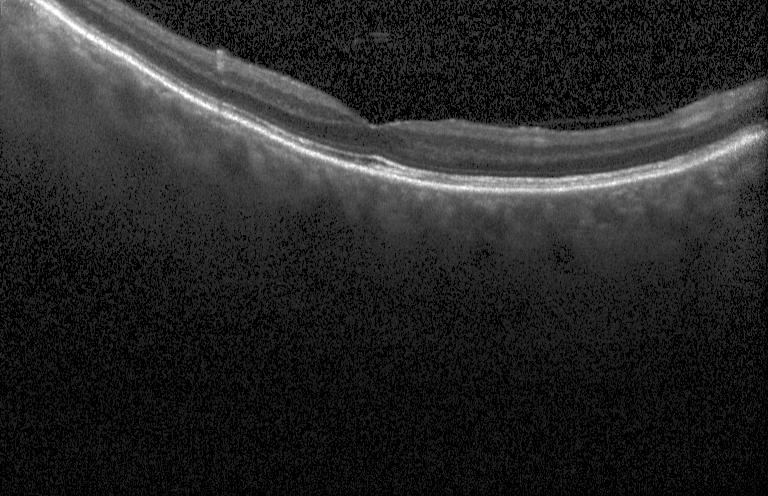
Acquired on a Heidelberg Spectralis · optical coherence tomography scan. Assessment: no choroidal neovascularization, no diabetic macular edema, and no drusen.